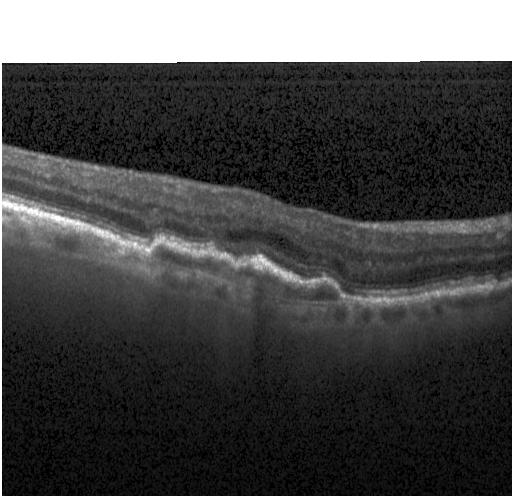

Optical coherence tomography B-scan, spectral-domain optical coherence tomography, Heidelberg Spectralis OCT system
Impression: a choroidal neovascular membrane.